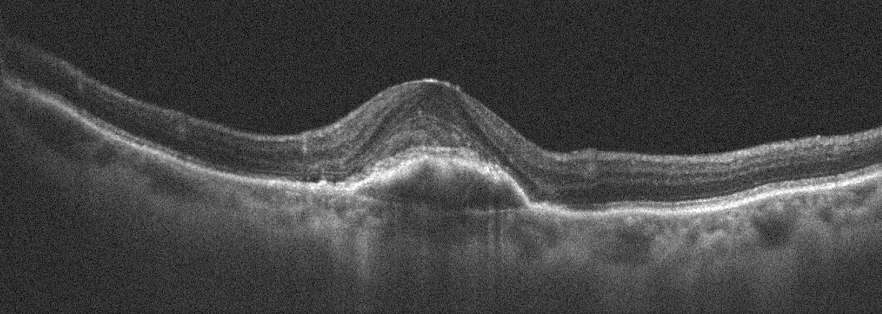

Acquired on an Optovue Avanti RTVue XR; macular scan; oculus sinister; OCT B-scan — Dx: age-related macular degeneration.